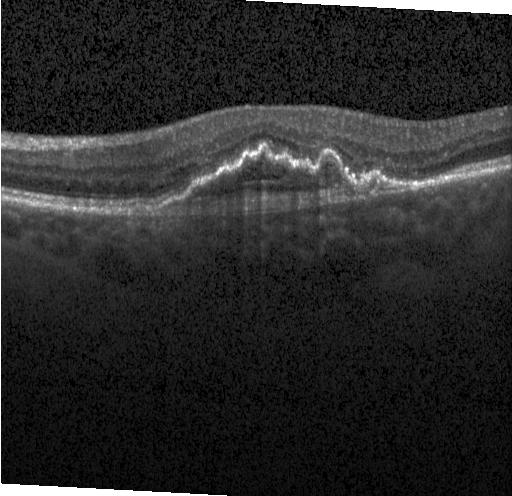 Optical coherence tomography B-scan.
The scan shows a choroidal neovascular membrane.